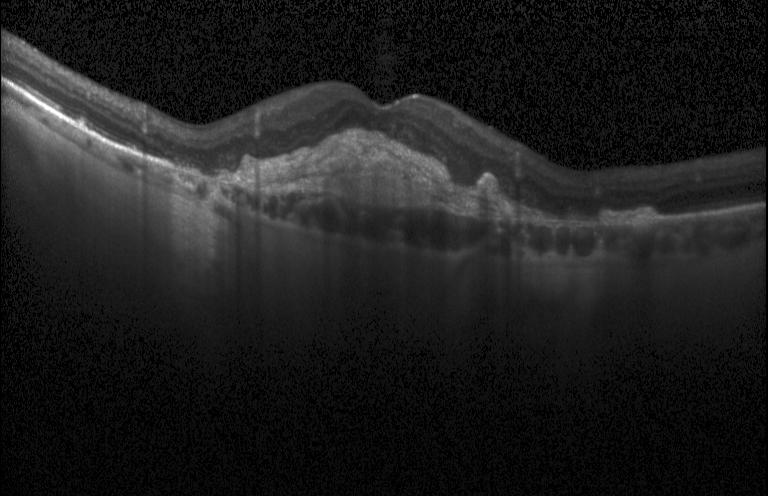
Optical coherence tomography scan
Assessment: CNV.